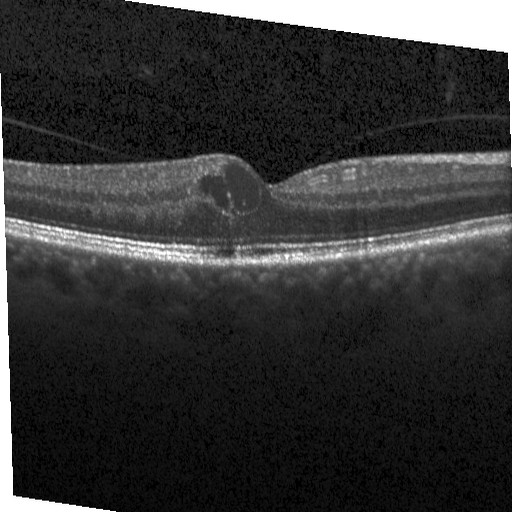

Through the macula. Spectral-domain OCT. Optical coherence tomography scan. Acquired on a Heidelberg Spectralis — This B-scan demonstrates diabetic macular edema.